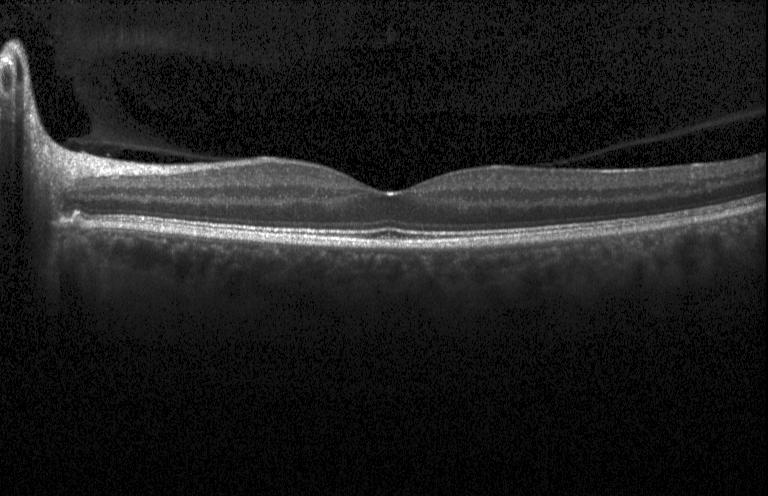

OCT B-scan showing no CNV, no DME, and no drusen.